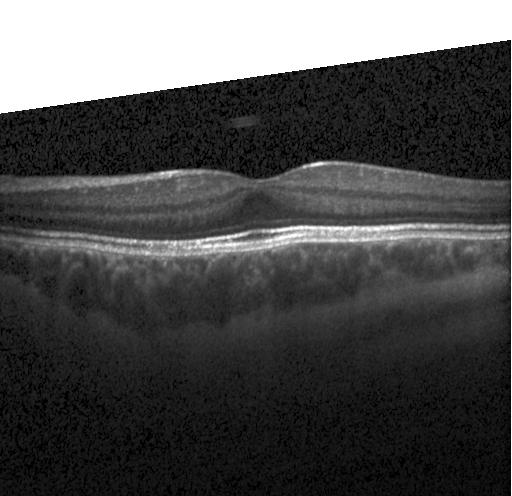 OCT line scan
Macular OCT: no evidence of choroidal neovascularization, diabetic macular edema, or drusen.